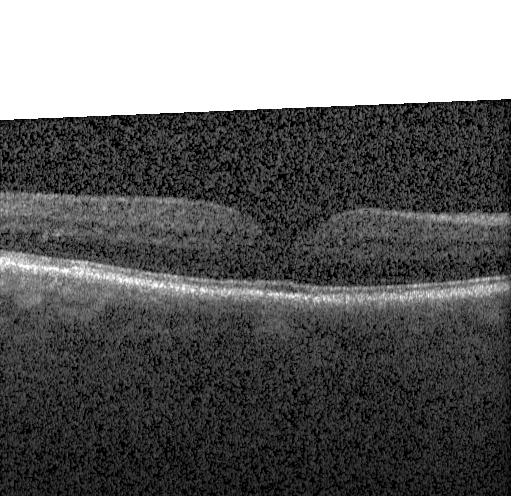 Optical coherence tomography scan — The scan shows no evidence of CNV, DME, or drusen.